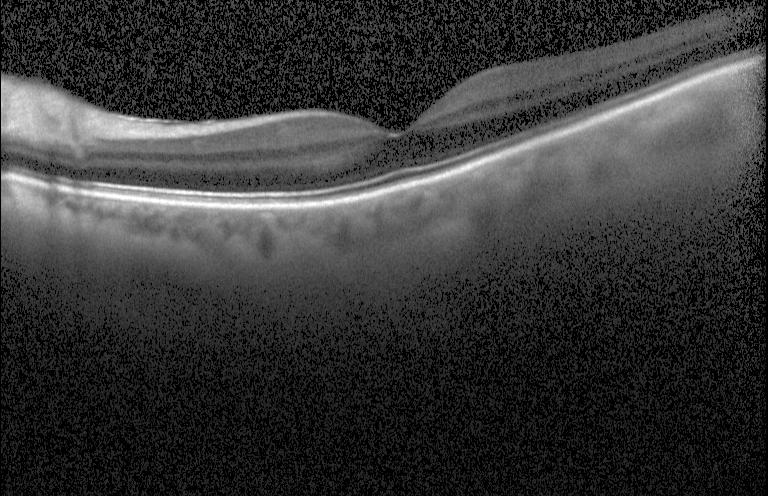
SD-OCT; retinal OCT B-scan.
Assessment: neither choroidal neovascularization, diabetic macular edema, nor drusen.